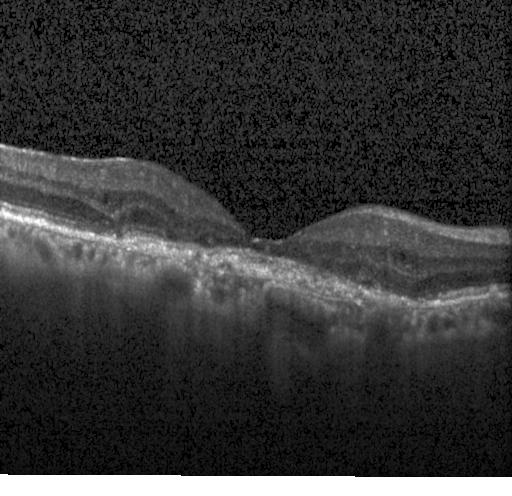
OCT B-scan showing a choroidal neovascular membrane.